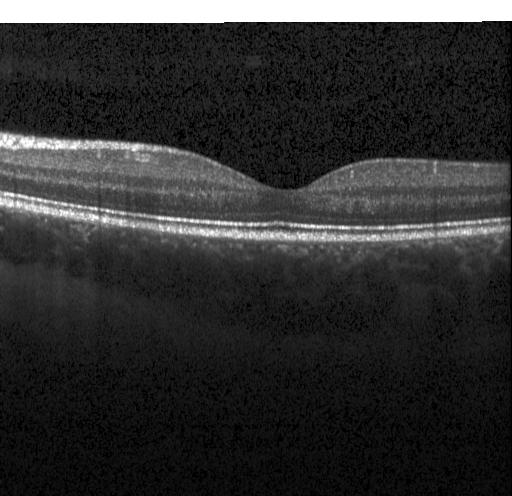 Optical coherence tomography B-scan.
Impression: no choroidal neovascularization, no diabetic macular edema, and no drusen.